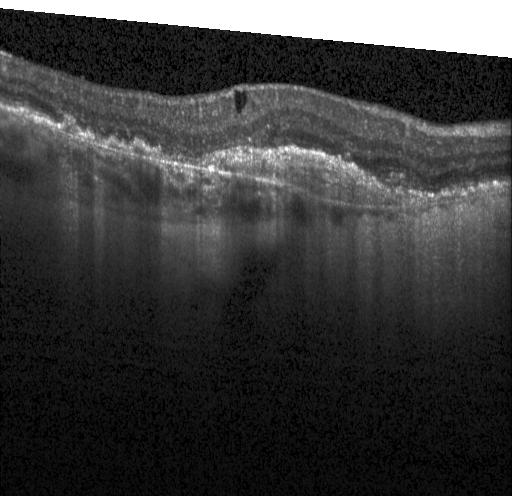

Retinal OCT cross-section, through the macula, Heidelberg Spectralis OCT system. Assessment: CNV.